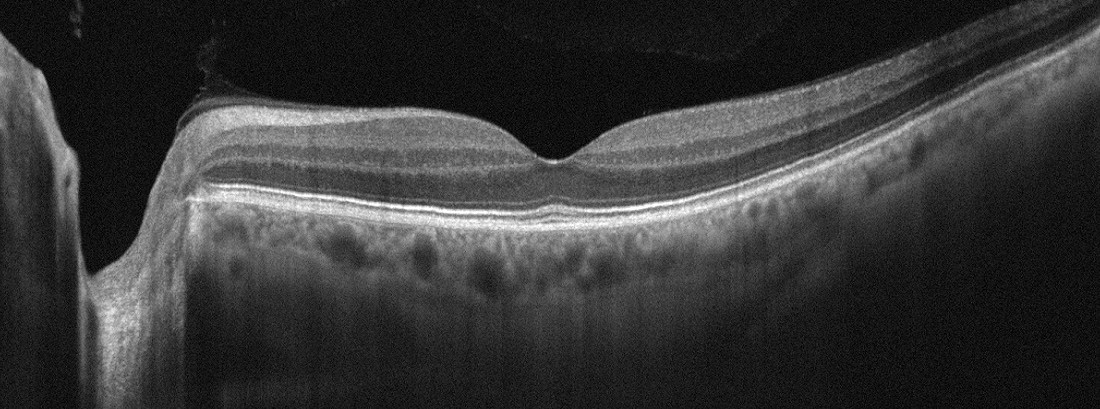
Absence of AMD, DME, ERM, RAO, RVO, and vitreomacular interface disease.